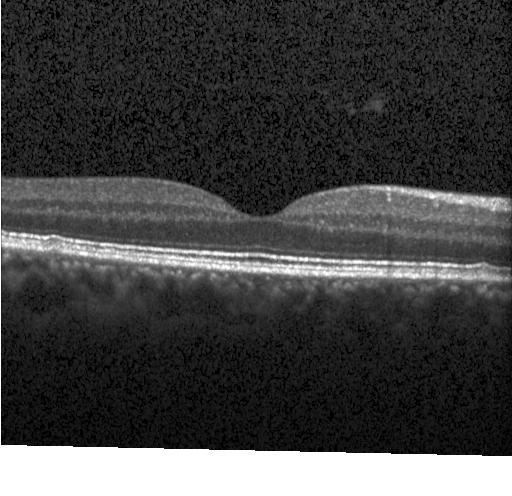 Dx: no CNV, DME, or drusen.